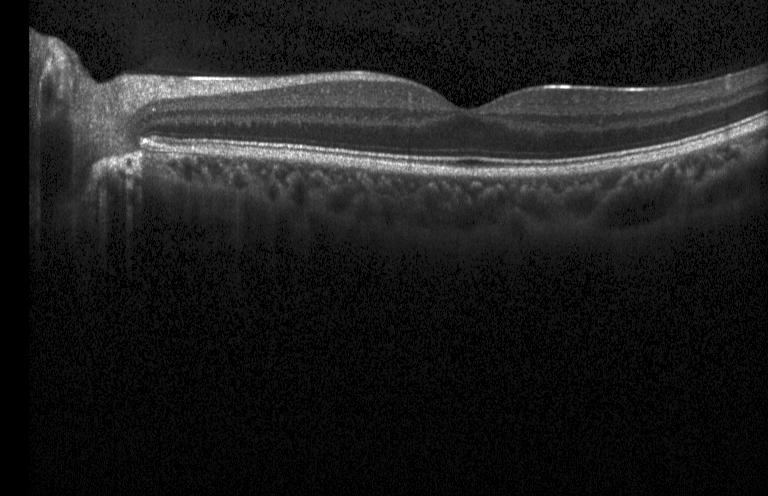

Retinal OCT cross-section
OCT finding: neither choroidal neovascularization, diabetic macular edema, nor drusen.